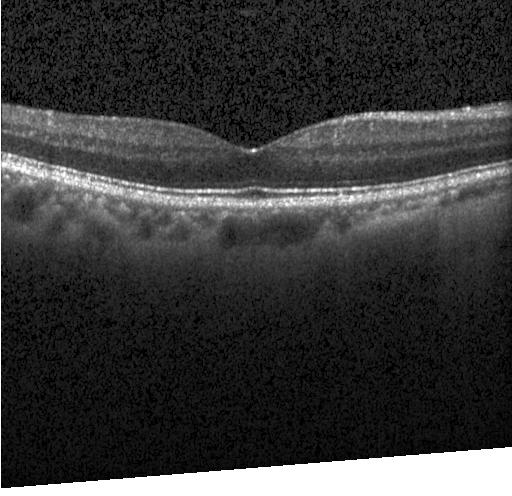

Through the macula · retinal OCT B-scan · SD-OCT — OCT finding: neither CNV, DME, nor drusen.